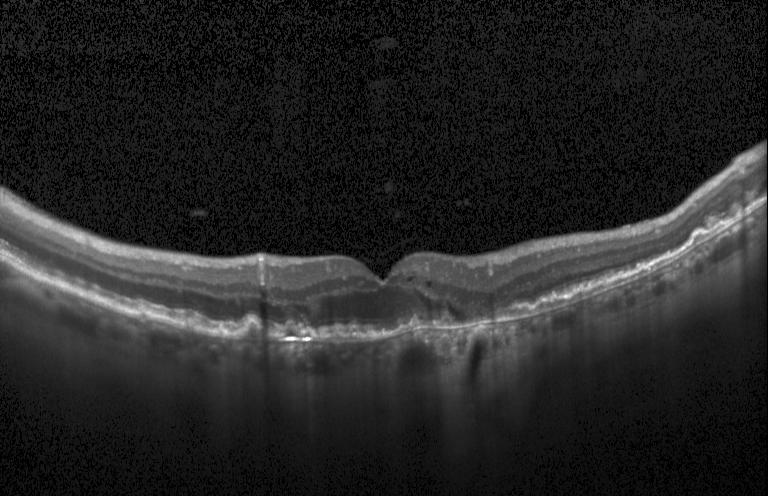 Optical coherence tomography B-scan
Assessment: a choroidal neovascular membrane.